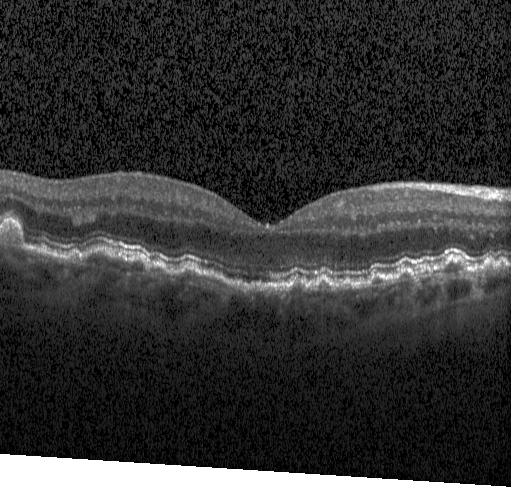

Optical coherence tomography B-scan. Horizontal scan through the fovea. Heidelberg Spectralis OCT system. Assessment: sub-RPE drusenoid deposits.